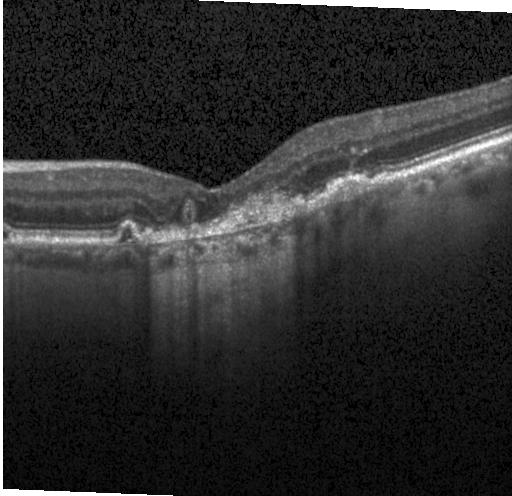 OCT B-scan; spectral-domain OCT — Finding: choroidal neovascularization (CNV).